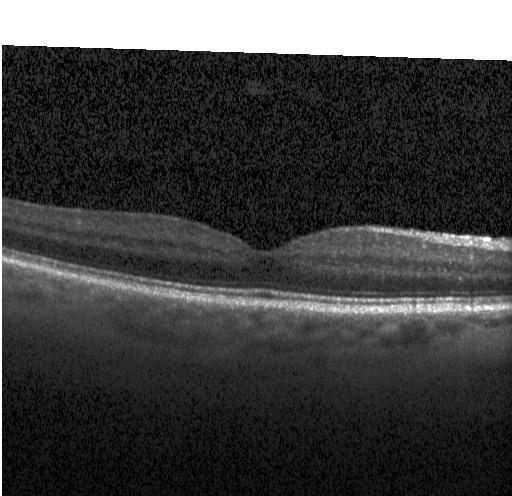
Finding: no CNV, no DME, and no drusen.